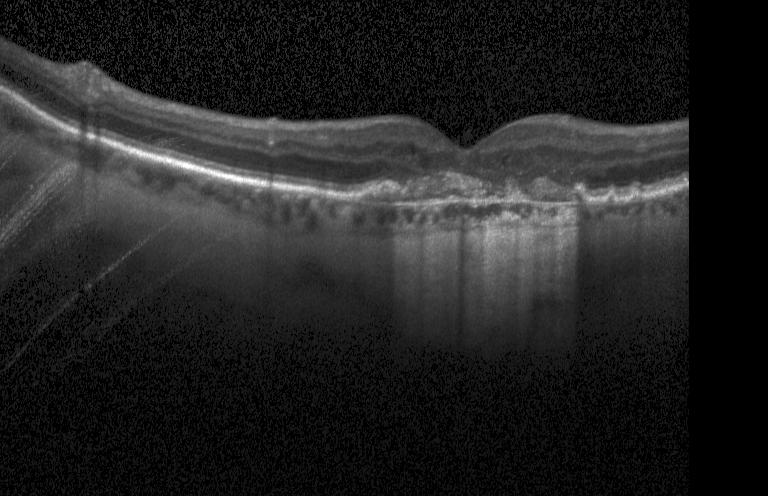
Optical coherence tomography scan. OCT finding: a choroidal neovascular membrane.